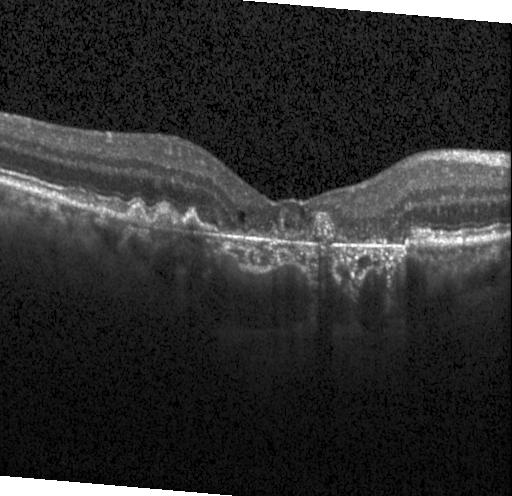

Diagnosis: a choroidal neovascular membrane.